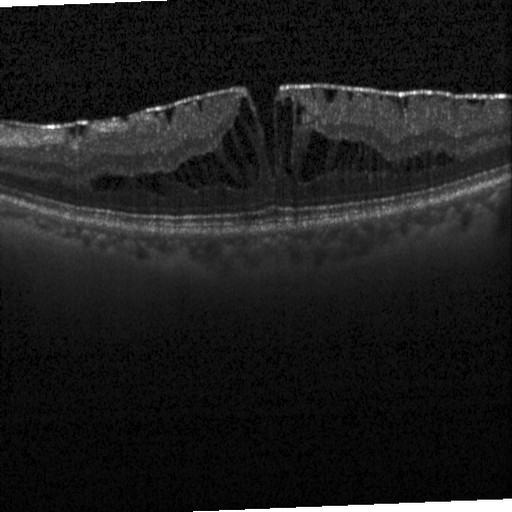
Through the macula; OCT line scan; Heidelberg Spectralis OCT system; spectral-domain optical coherence tomography
Impression: diabetic macular edema (DME).